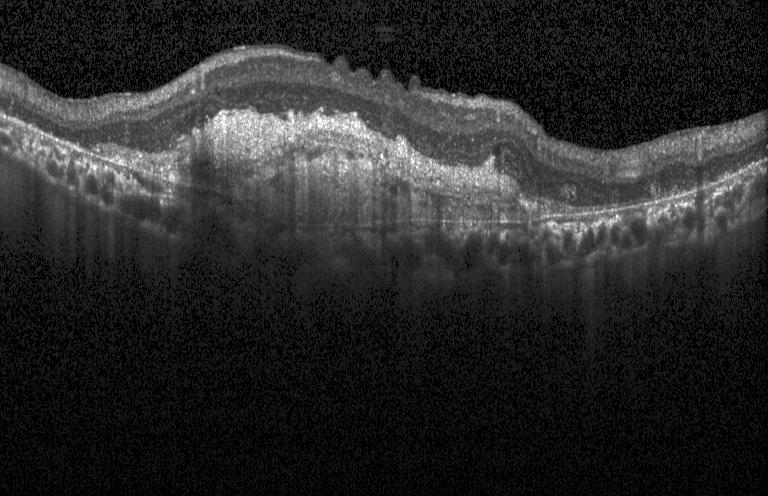
Heidelberg Spectralis OCT system; spectral-domain optical coherence tomography; retinal OCT cross-section
The scan shows a choroidal neovascular membrane.